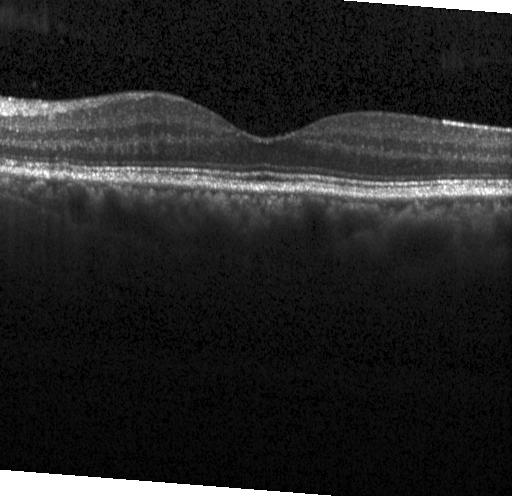

Heidelberg Spectralis OCT system · SD-OCT · optical coherence tomography scan · macular scan. The scan shows no evidence of choroidal neovascularization, diabetic macular edema, or drusen.